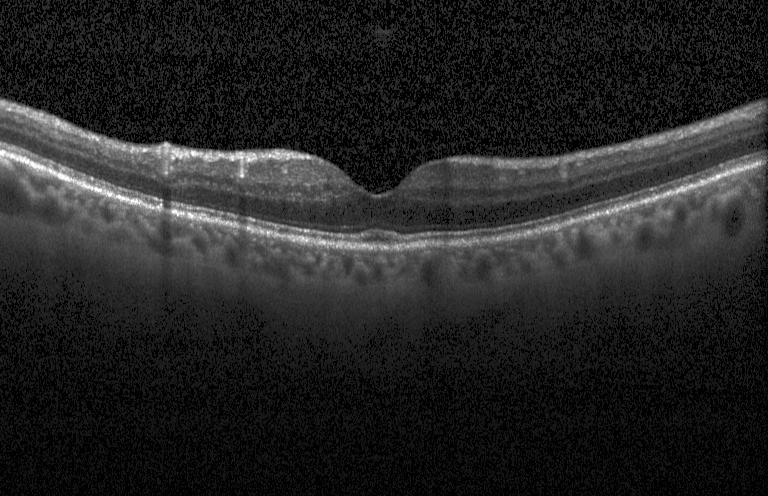
Diagnosis: no choroidal neovascularization, no diabetic macular edema, and no drusen.